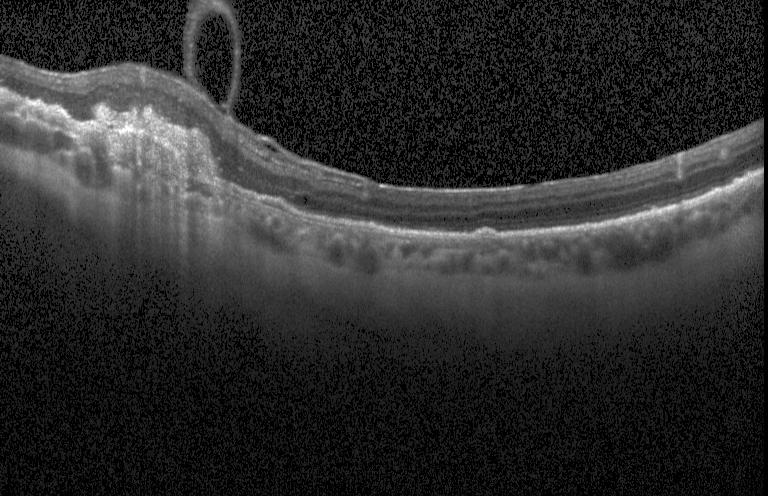

Dx: a choroidal neovascular membrane.